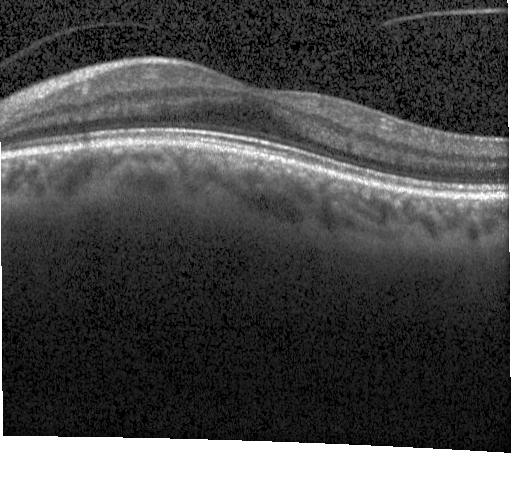 Assessment: no evidence of CNV, DME, or drusen.